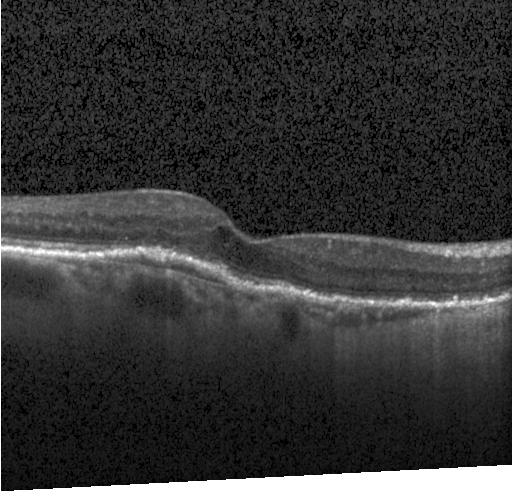
Retinal OCT B-scan.
Macular OCT: a choroidal neovascular membrane.